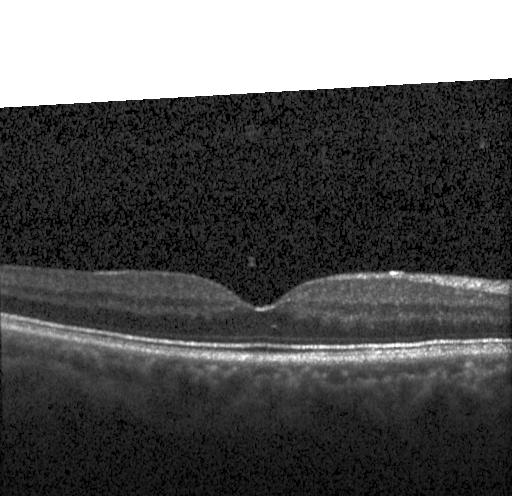 Optical coherence tomography scan
No choroidal neovascularization, diabetic macular edema, or drusen.